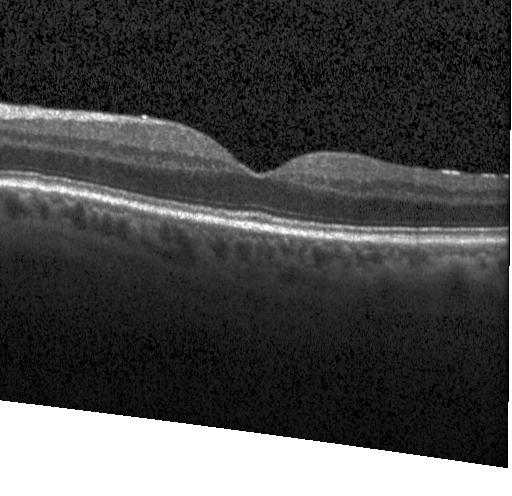

Heidelberg Spectralis OCT system · macular scan · retinal OCT cross-section · spectral-domain optical coherence tomography.
Macular OCT: no evidence of choroidal neovascularization, diabetic macular edema, or drusen.